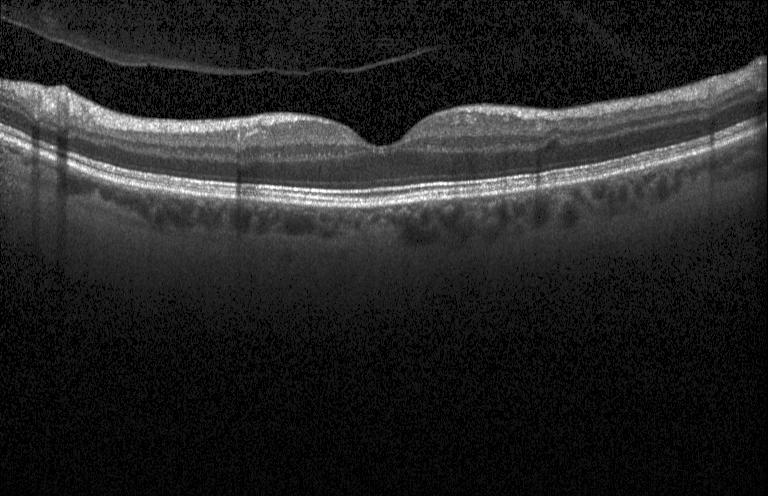
OCT B-scan. Macular scan
Dx: no CNV, DME, or drusen.